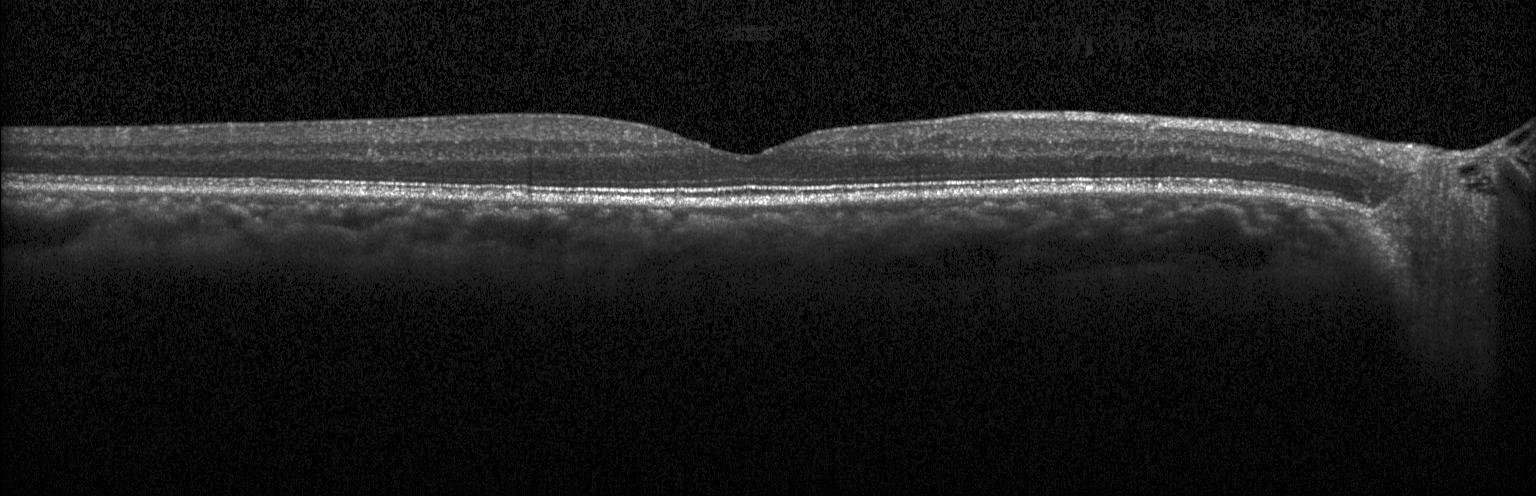

Assessment: neither CNV, DME, nor drusen.